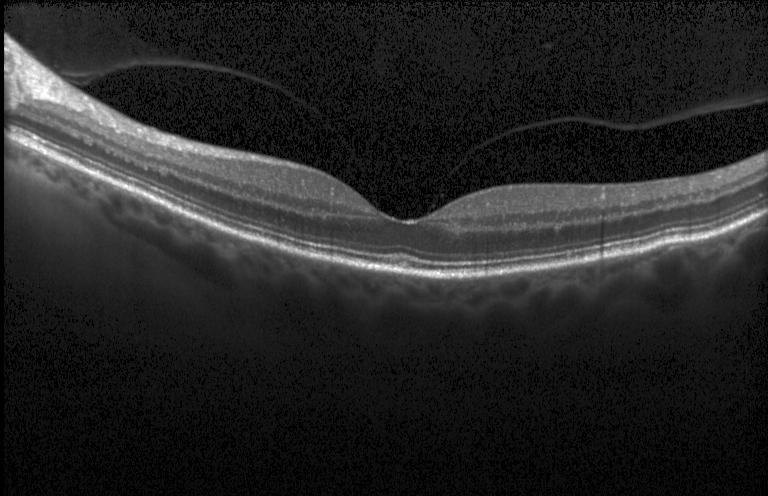 Assessment: no evidence of choroidal neovascularization, diabetic macular edema, or drusen.